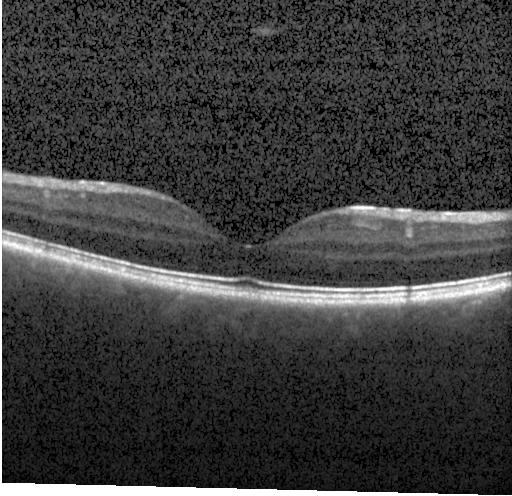 Heidelberg Spectralis OCT system. Retinal OCT cross-section. Through the macula
Finding: no CNV, DME, or drusen.